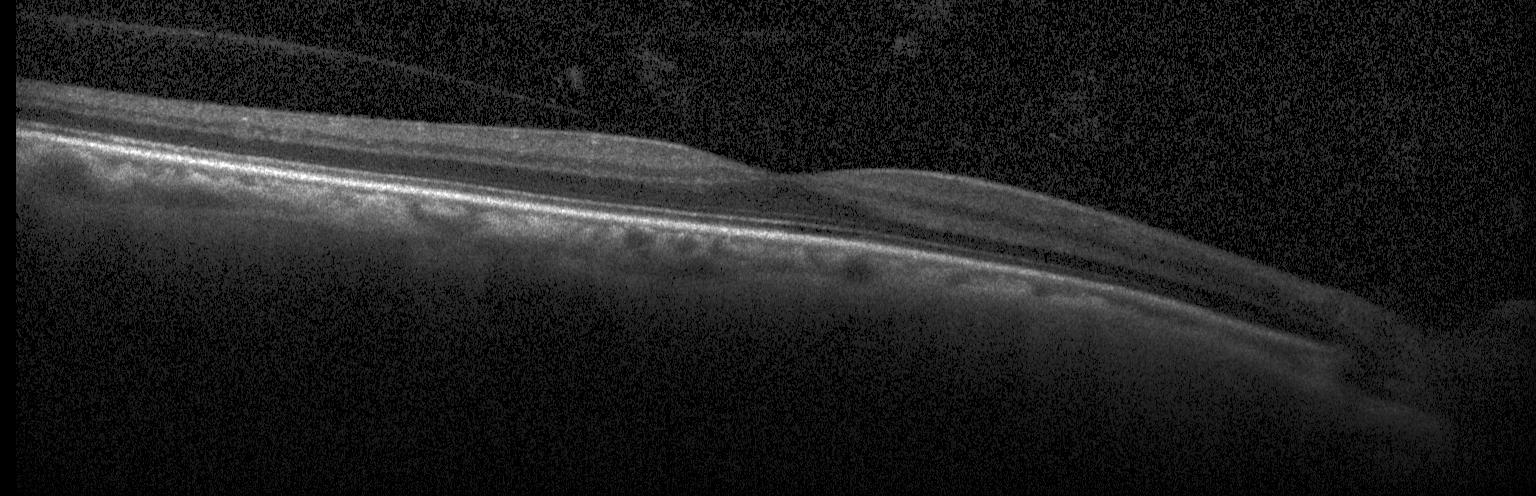
OCT line scan, instrument: Heidelberg Spectralis.
Assessment: no choroidal neovascularization, no diabetic macular edema, and no drusen.